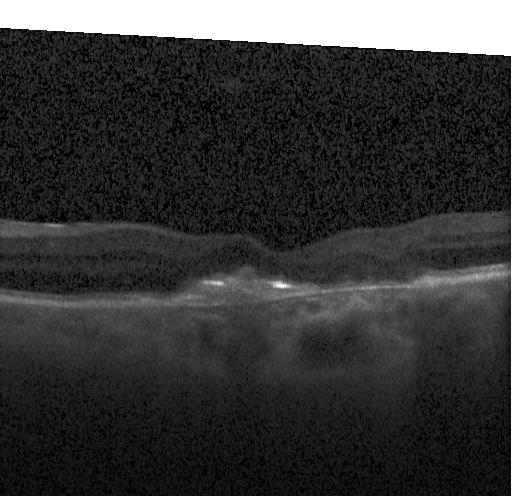 SD-OCT. Centered on the fovea. OCT B-scan. Acquired on a Heidelberg Spectralis — Finding: choroidal neovascularization.